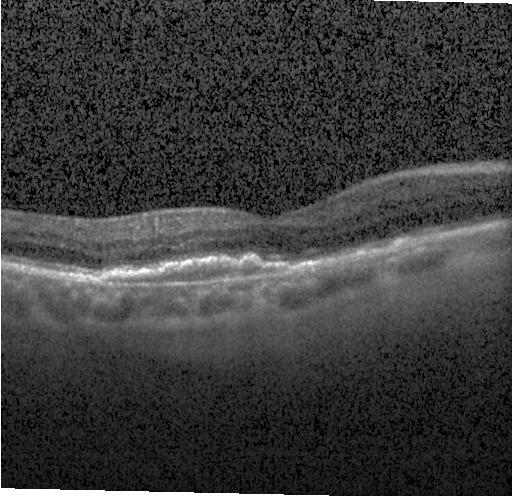
Optical coherence tomography B-scan — Finding: a choroidal neovascular membrane.